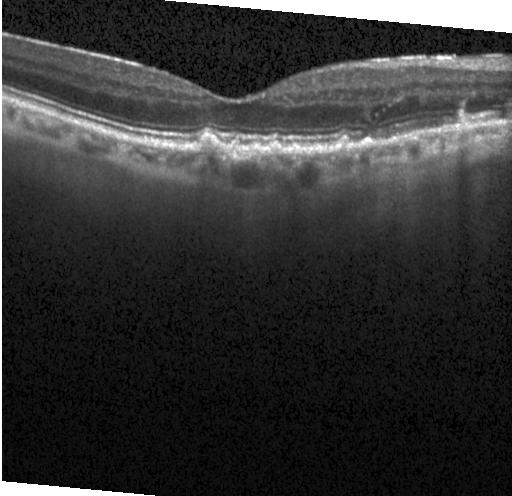
Diagnosis: multiple drusen.